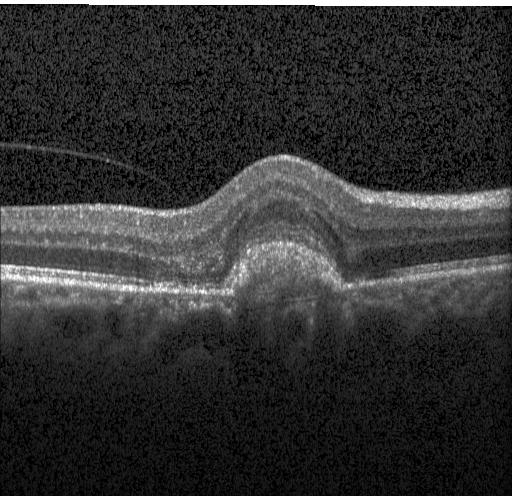

Heidelberg Spectralis, horizontal scan through the fovea, spectral-domain OCT, retinal OCT cross-section. Assessment: CNV.